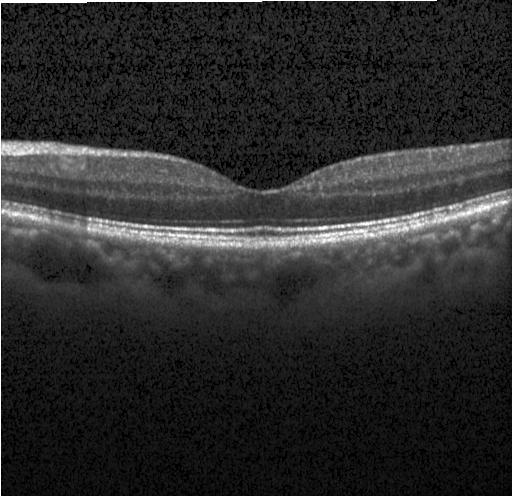

Dx: no CNV, no DME, and no drusen.